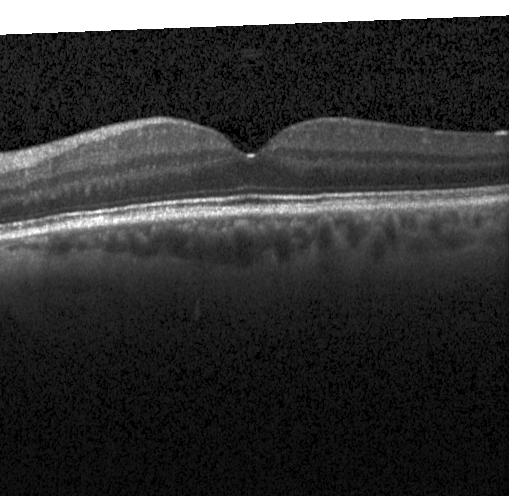
OCT line scan. Centered on the fovea. Spectral-domain OCT. Instrument: Heidelberg Spectralis
OCT finding: no evidence of CNV, DME, or drusen.